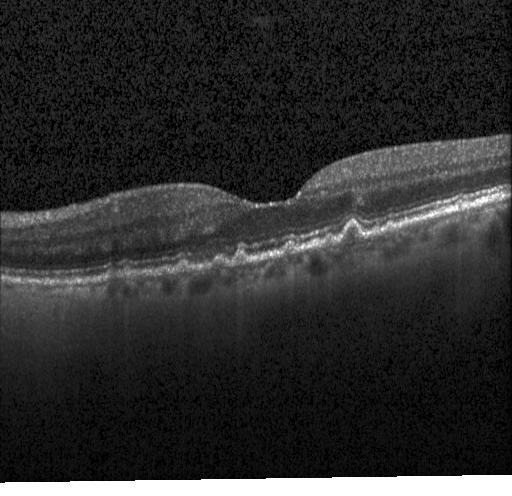

Assessment: drusen.